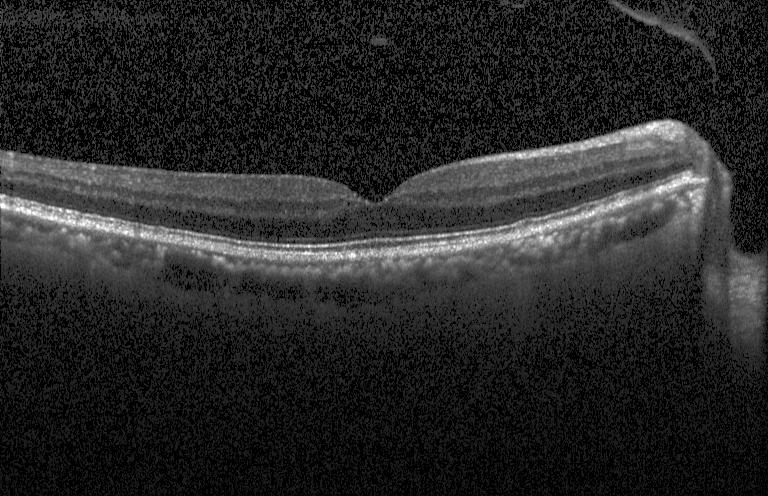

Through the macula, OCT line scan, spectral-domain optical coherence tomography.
The scan shows no CNV, no DME, and no drusen.